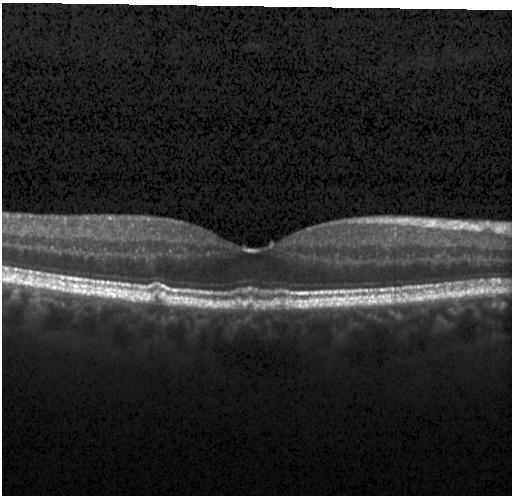

Optical coherence tomography B-scan. Heidelberg Spectralis. Horizontal scan through the fovea — Impression: drusen.